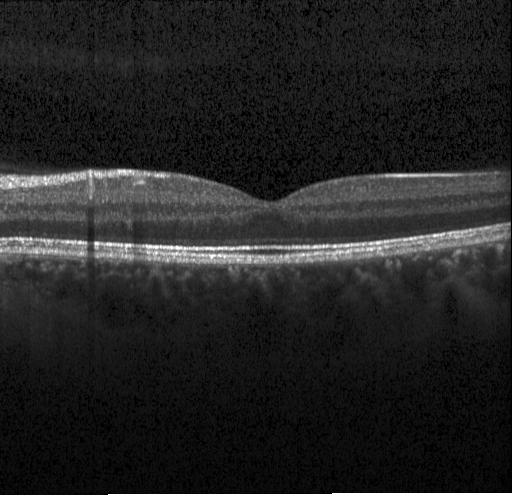 Spectral-domain optical coherence tomography; through the macula; retinal OCT cross-section
Impression: no choroidal neovascularization, diabetic macular edema, or drusen.